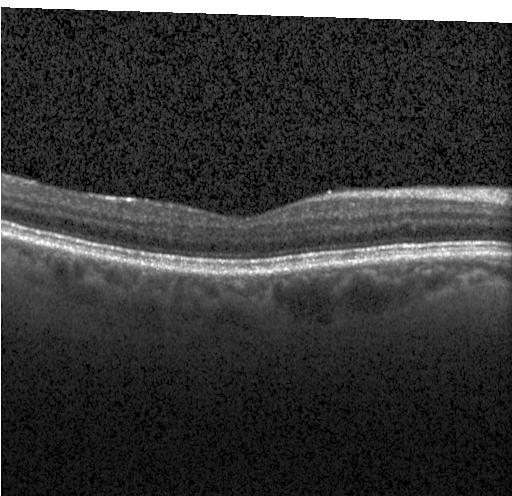 Retinal OCT cross-section showing no CNV, no DME, and no drusen.